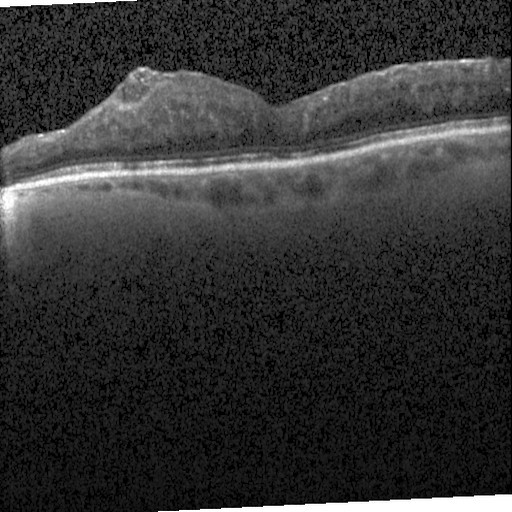

Instrument: Heidelberg Spectralis. Retinal OCT cross-section. SD-OCT.
Diabetic macular edema.